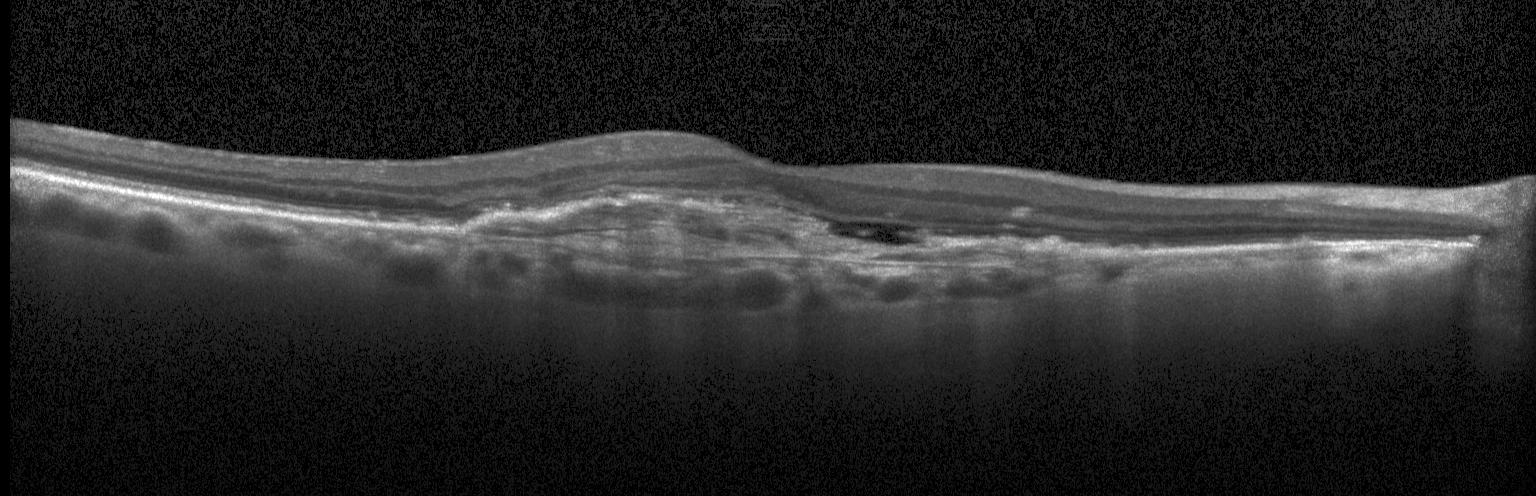 Optical coherence tomography B-scan · SD-OCT · fovea-centered · Heidelberg Spectralis OCT system
Macular OCT: CNV.